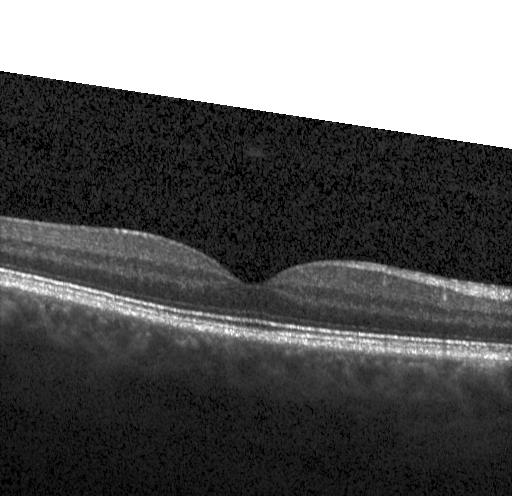

Spectral-domain OCT B-scan: neither CNV, DME, nor drusen.